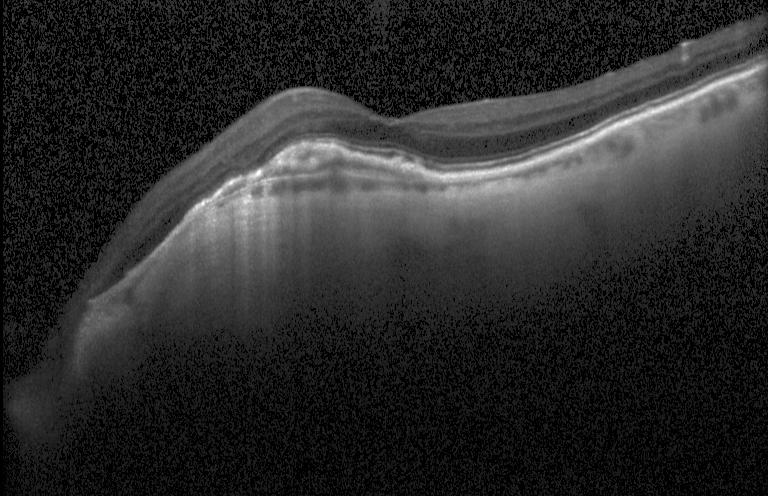
Heidelberg Spectralis OCT system. Horizontal scan through the fovea. Optical coherence tomography B-scan. SD-OCT.
Dx: choroidal neovascularization.